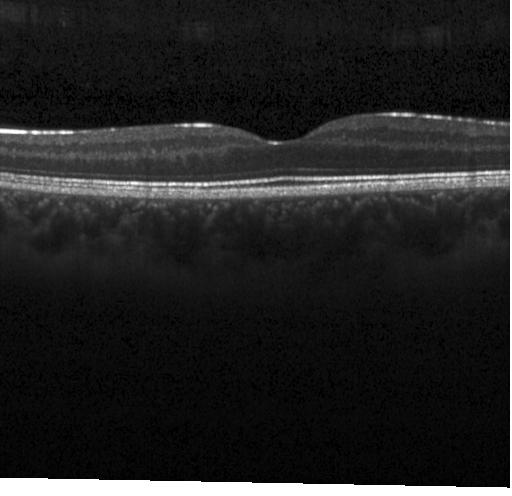

Macular OCT: no choroidal neovascularization, no diabetic macular edema, and no drusen.